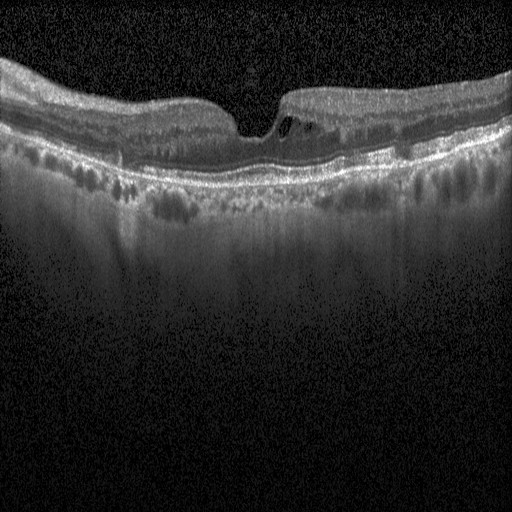
OCT line scan. Finding: diabetic macular edema (DME).